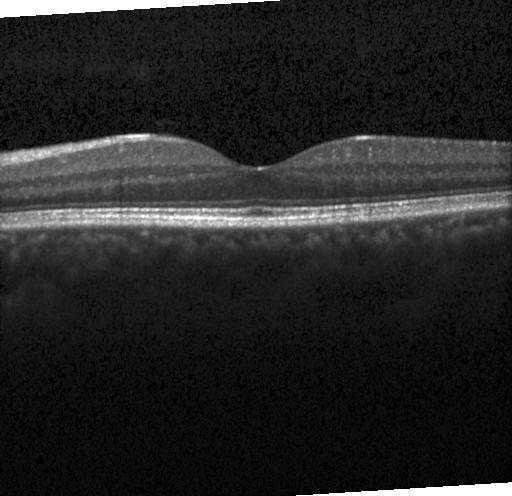 Optical coherence tomography B-scan. SD-OCT
Diagnosis: neither choroidal neovascularization, diabetic macular edema, nor drusen.